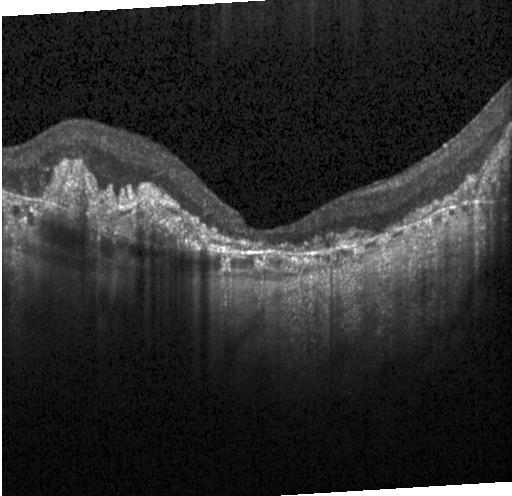

Spectral-domain OCT · retinal OCT B-scan.
Impression: choroidal neovascularization.